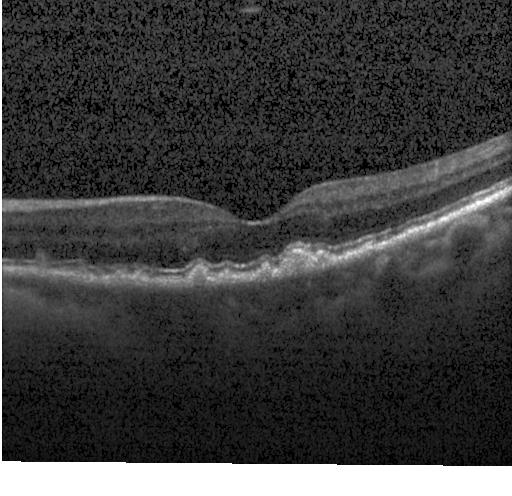

Retinal OCT B-scan — Diagnosis: sub-RPE drusenoid deposits.